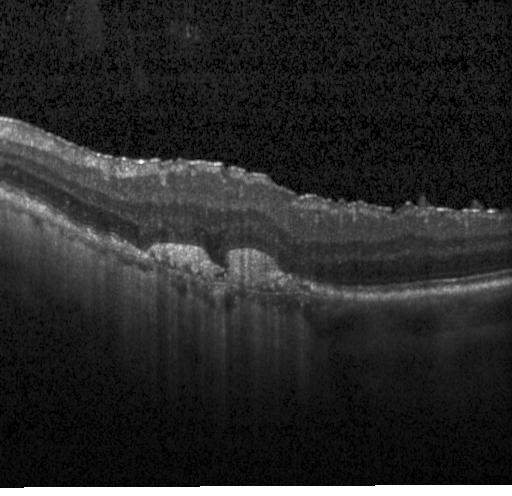

A choroidal neovascular membrane.